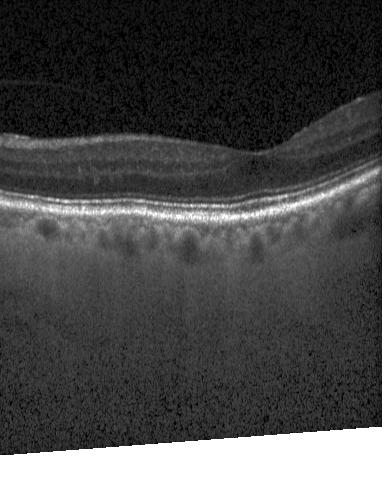 Instrument: Heidelberg Spectralis; optical coherence tomography B-scan; macular scan.
OCT finding: neither CNV, DME, nor drusen.